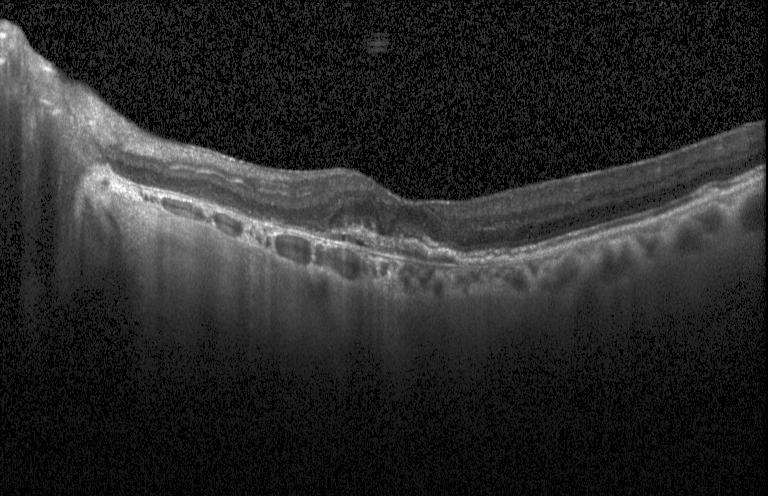
Diagnosis: a choroidal neovascular membrane.